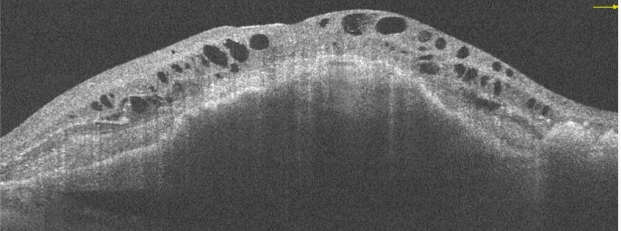
OCT line scan
The scan shows AMD.